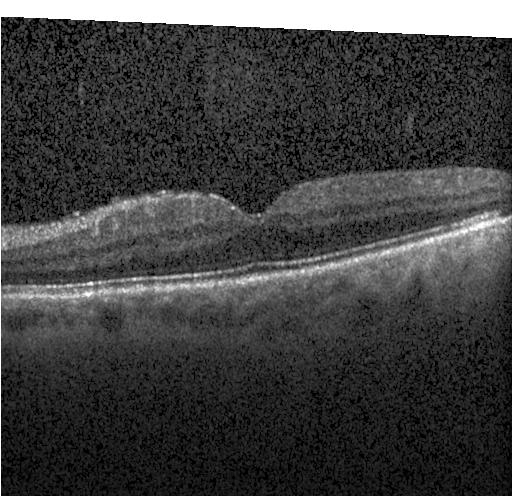
Heidelberg Spectralis, optical coherence tomography B-scan, centered on the fovea
Impression: neither choroidal neovascularization, diabetic macular edema, nor drusen.